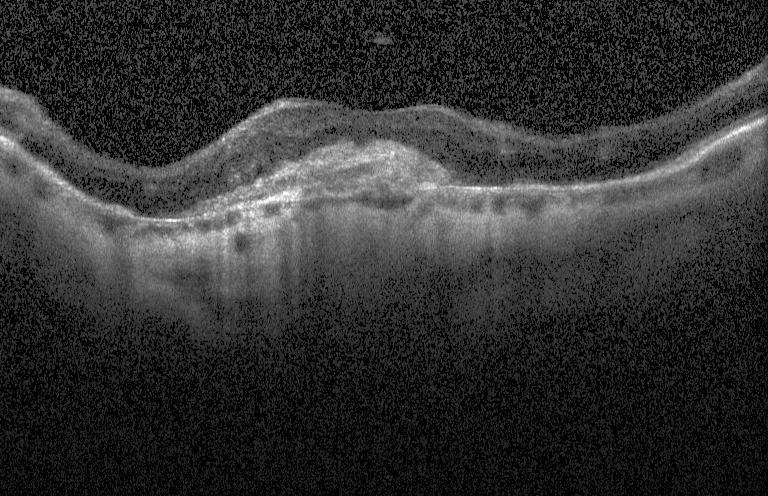
Assessment: a choroidal neovascular membrane.